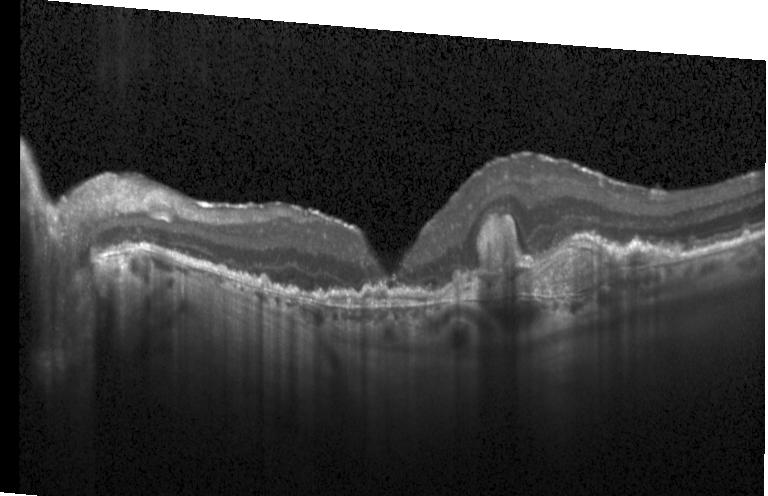
Finding: choroidal neovascularization.